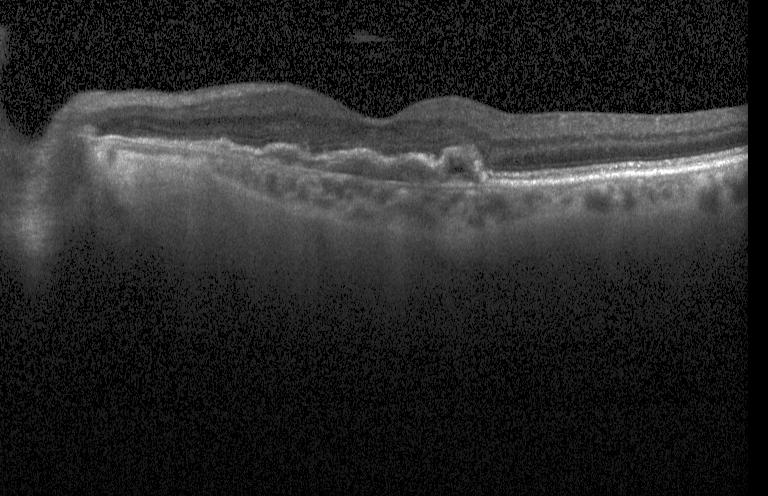
OCT line scan.
Diagnosis: a choroidal neovascular membrane.